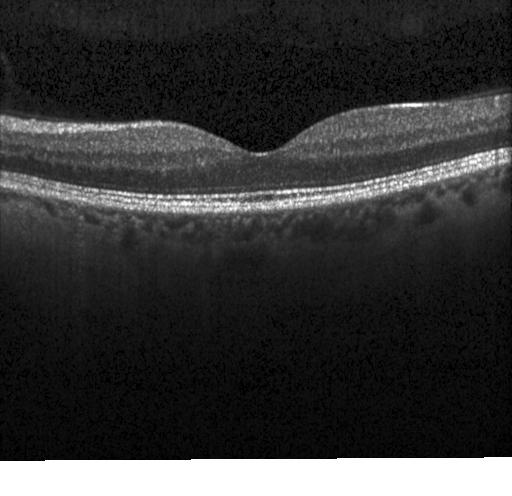
Heidelberg Spectralis · retinal OCT cross-section · macular scan
Impression: no evidence of CNV, DME, or drusen.